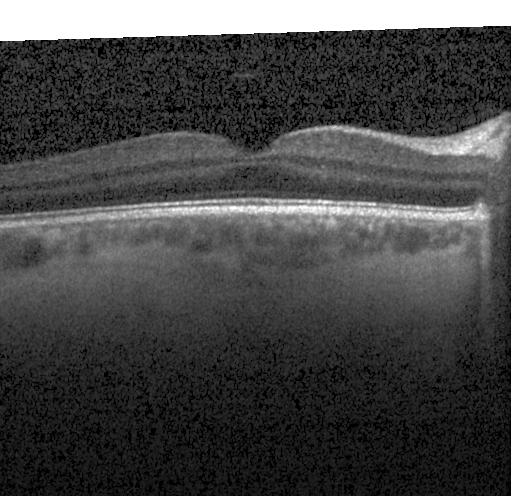 Retinal OCT B-scan. This B-scan demonstrates no evidence of choroidal neovascularization, diabetic macular edema, or drusen.